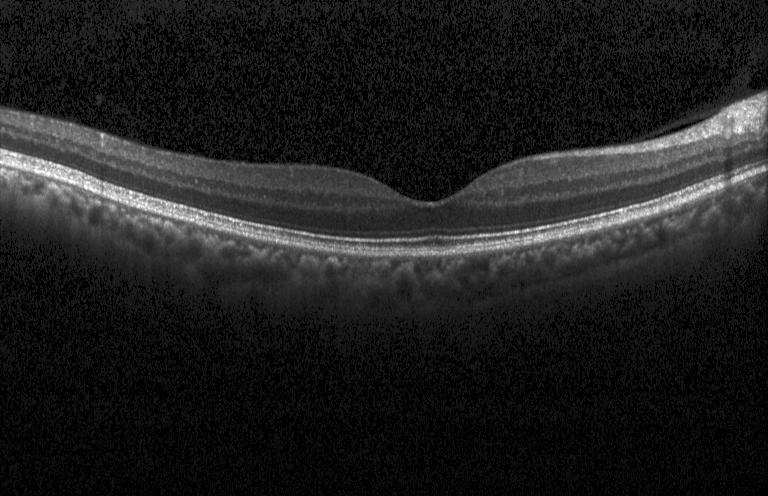
Impression: no CNV, DME, or drusen.